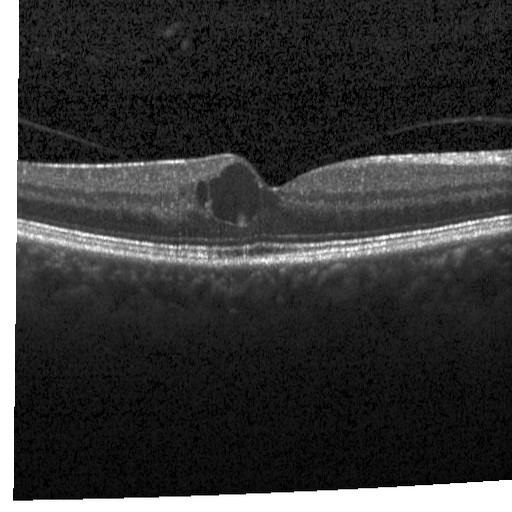
Spectral-domain optical coherence tomography, Heidelberg Spectralis OCT system, retinal OCT cross-section. This B-scan demonstrates diabetic macular edema (DME).